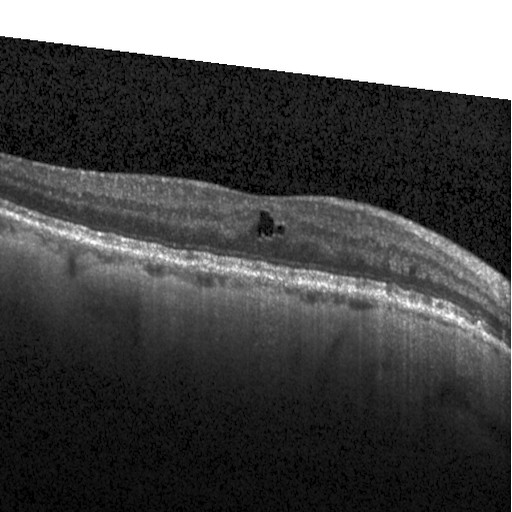

Macular scan; OCT line scan. The scan shows diabetic macular edema.